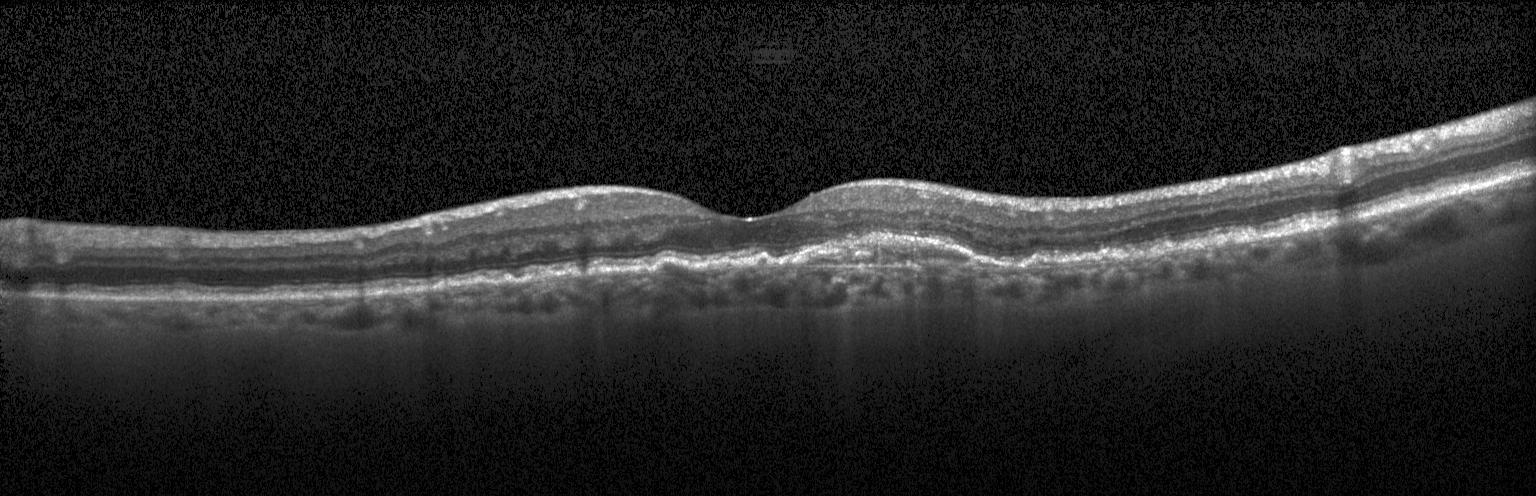
Instrument: Heidelberg Spectralis. Optical coherence tomography scan. SD-OCT. Horizontal scan through the fovea — Diagnosis: choroidal neovascularization (CNV).